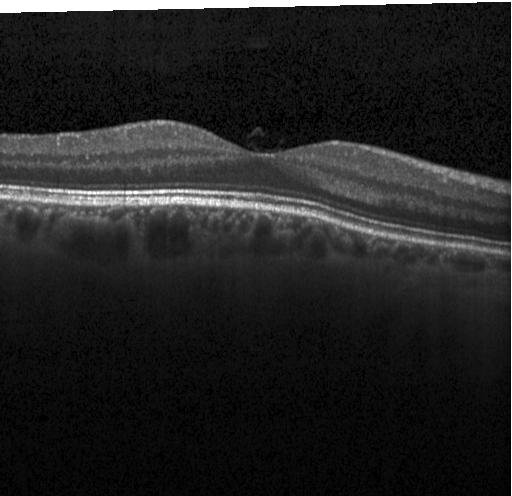

Optical coherence tomography B-scan. Assessment: no choroidal neovascularization, diabetic macular edema, or drusen.